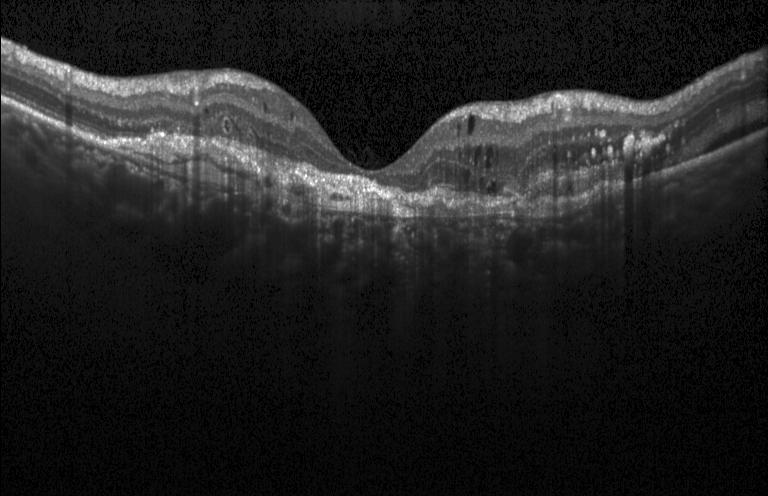

Assessment: a choroidal neovascular membrane.